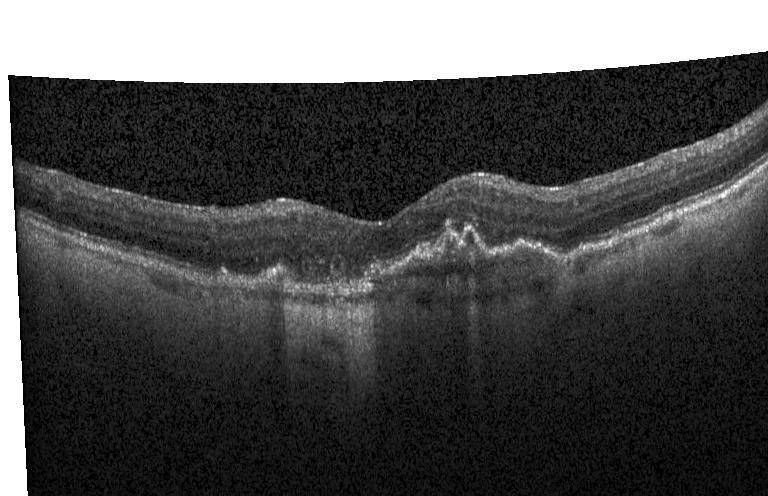

OCT B-scan, macular scan, instrument: Heidelberg Spectralis
Impression: a choroidal neovascular membrane.